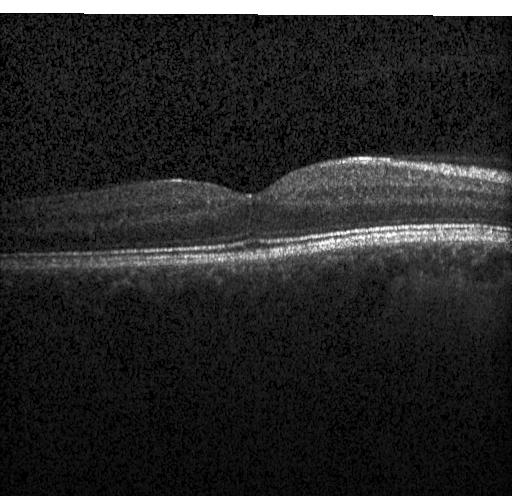
Impression: no choroidal neovascularization, no diabetic macular edema, and no drusen.